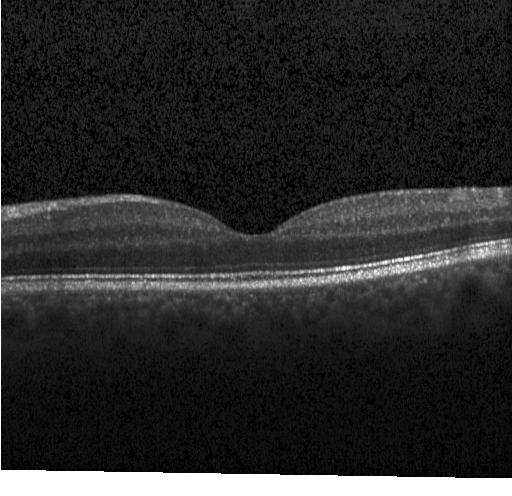

Spectral-domain optical coherence tomography; retinal OCT cross-section; centered on the fovea; acquired on a Heidelberg Spectralis.
OCT finding: no evidence of CNV, DME, or drusen.